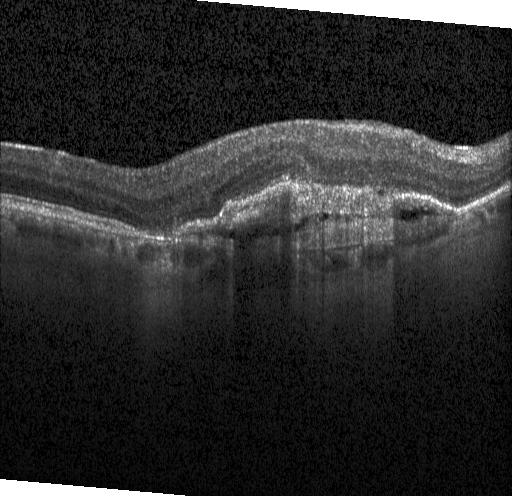 Retinal OCT B-scan
Diagnosis: a choroidal neovascular membrane.